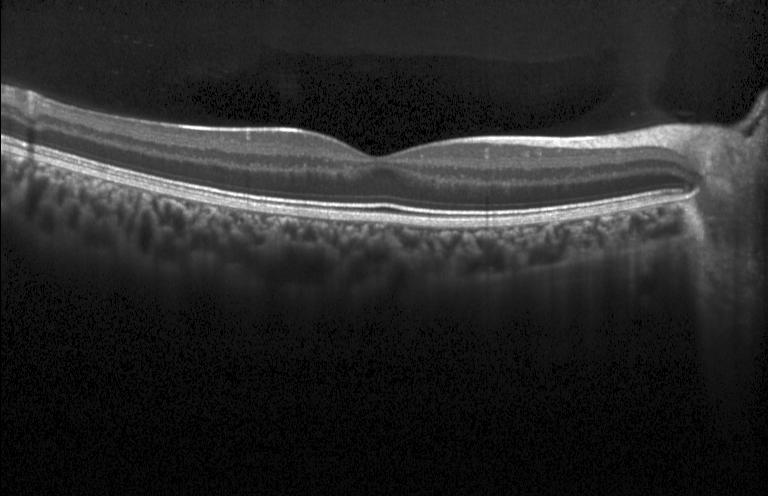 Acquired on a Heidelberg Spectralis · fovea-centered · optical coherence tomography B-scan.
Diagnosis: no choroidal neovascularization, diabetic macular edema, or drusen.